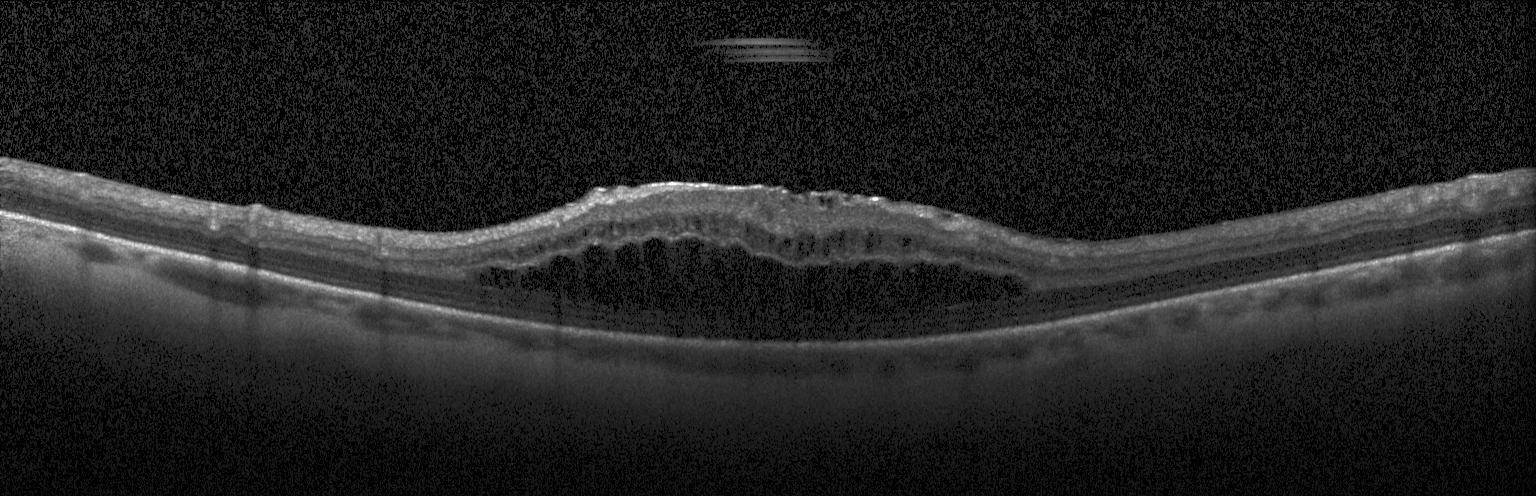
OCT line scan. Diabetic macular edema (DME).